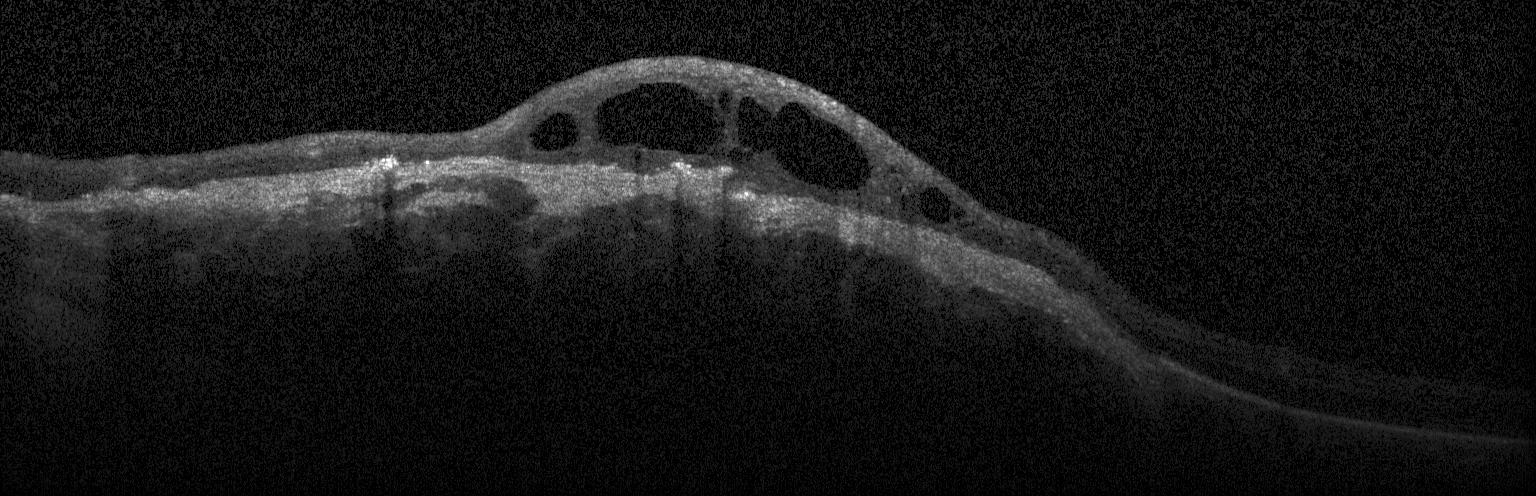
Macular OCT: choroidal neovascularization.